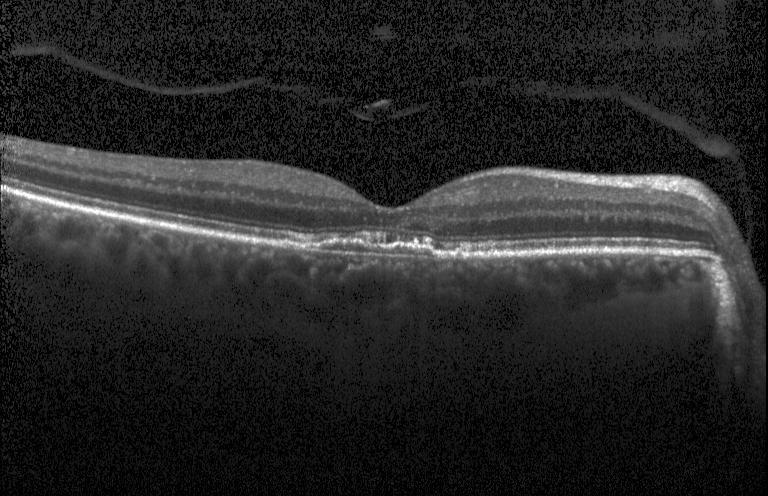 Centered on the fovea · OCT B-scan · acquired on a Heidelberg Spectralis · SD-OCT. Impression: choroidal neovascularization.